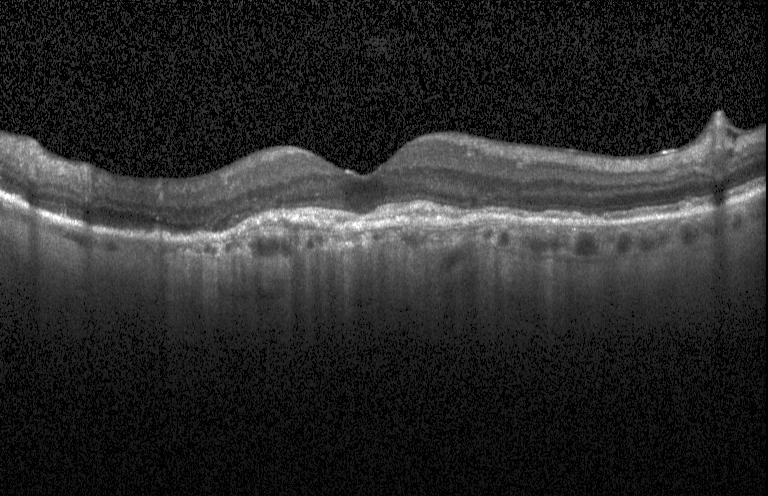

Diagnosis: a choroidal neovascular membrane.